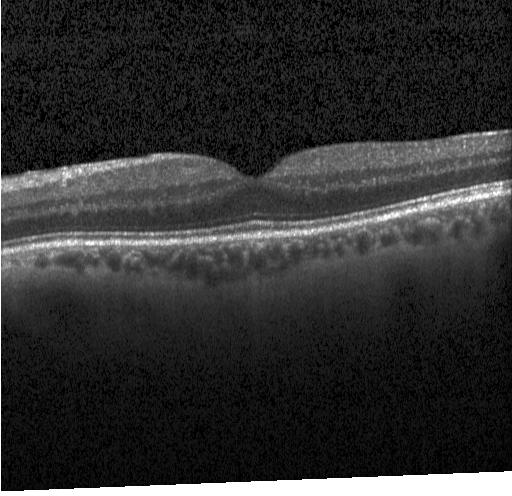
Impression: no CNV, no DME, and no drusen.